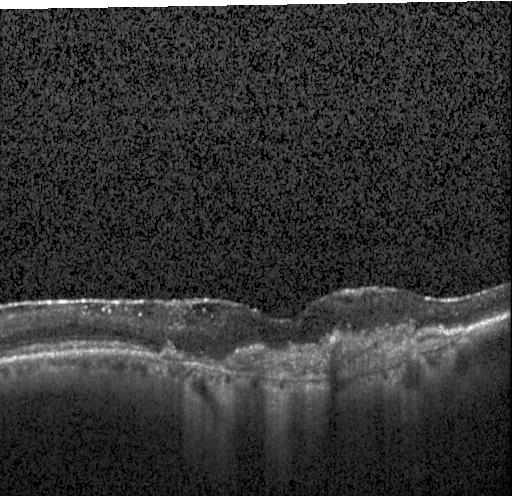 OCT scan showing choroidal neovascularization (CNV).